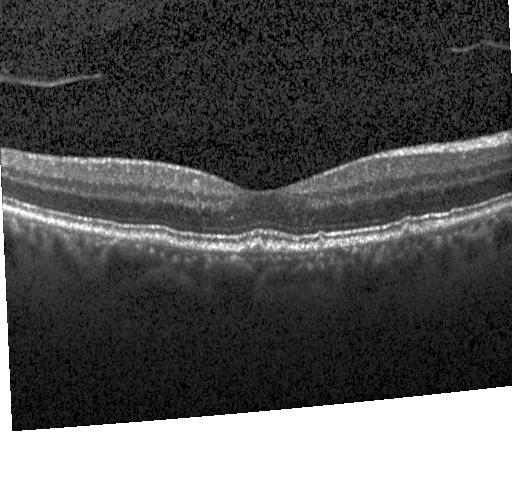 Optical coherence tomography scan
Diagnosis: sub-RPE drusenoid deposits.